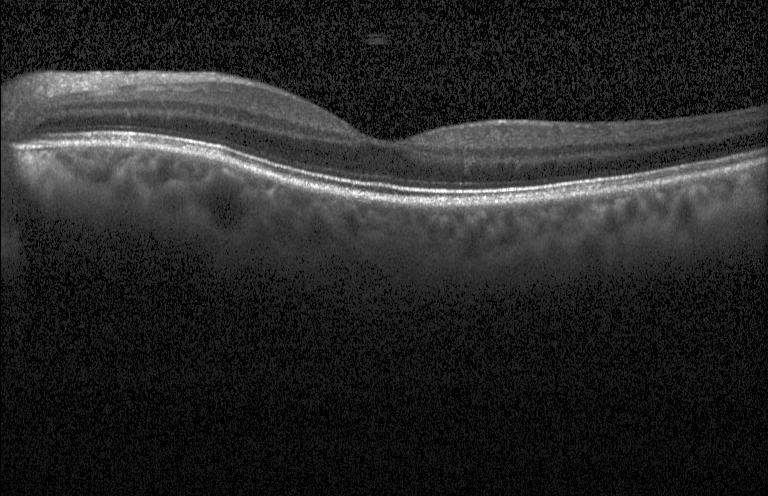

The scan shows no choroidal neovascularization, no diabetic macular edema, and no drusen.